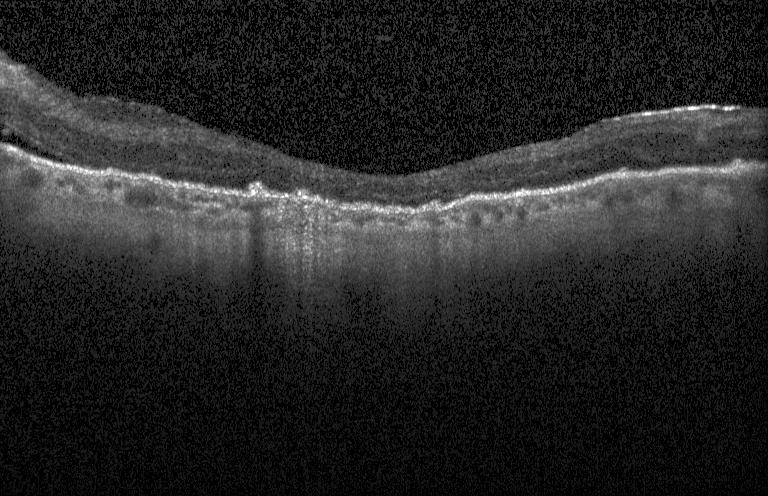

Fovea-centered. Spectral-domain optical coherence tomography. OCT line scan. Instrument: Heidelberg Spectralis — Assessment: choroidal neovascularization (CNV).